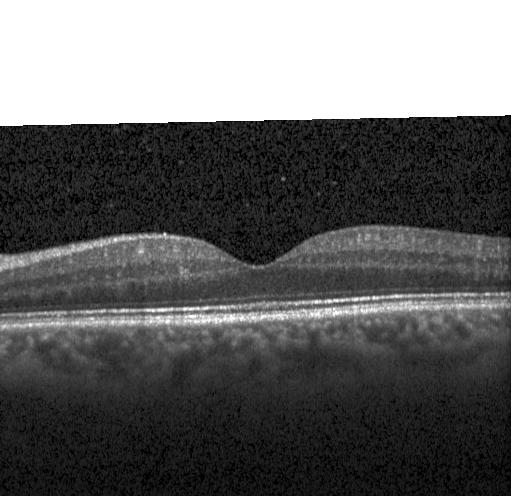 Retinal OCT cross-section.
Impression: no choroidal neovascularization, diabetic macular edema, or drusen.